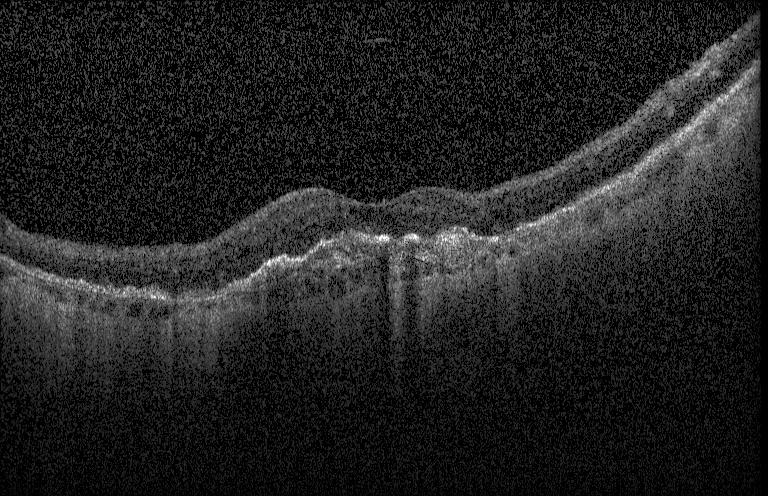
Acquired on a Heidelberg Spectralis · optical coherence tomography B-scan. OCT finding: a choroidal neovascular membrane.